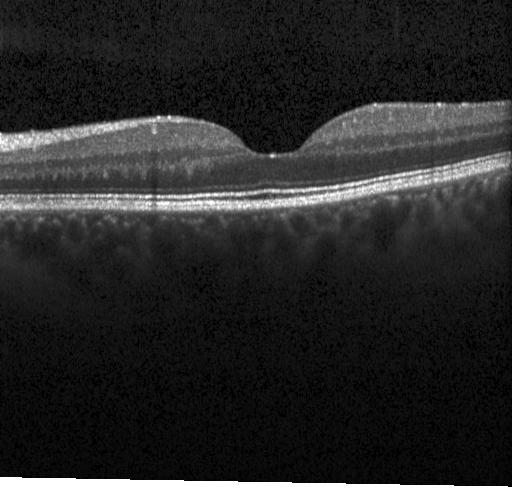

Optical coherence tomography scan. Spectral-domain OCT
Dx: no evidence of choroidal neovascularization, diabetic macular edema, or drusen.